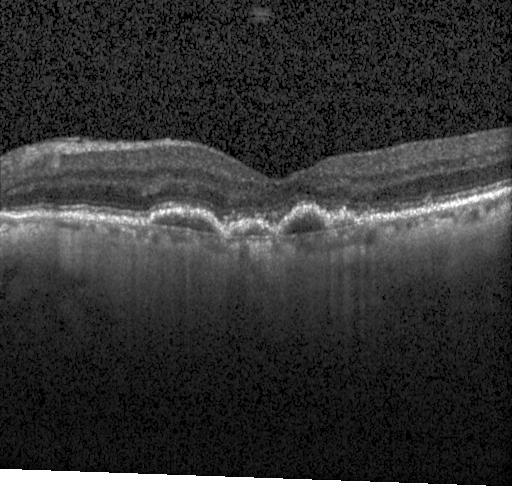

Acquired on a Heidelberg Spectralis. SD-OCT. OCT B-scan. OCT finding: a choroidal neovascular membrane.